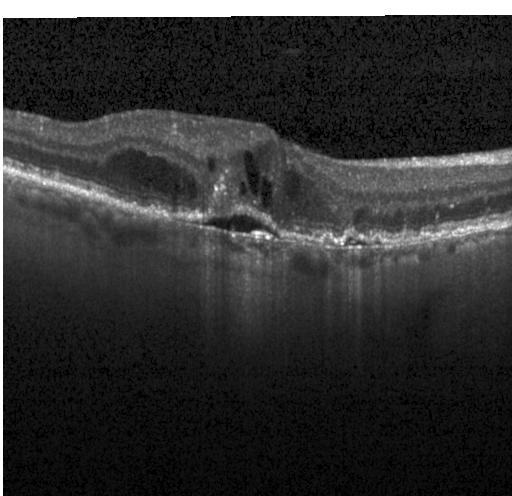
Macular OCT demonstrating a choroidal neovascular membrane.